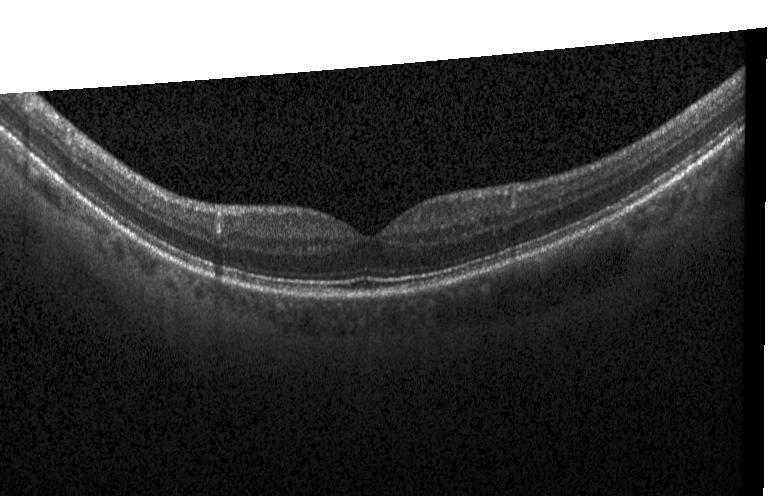
Retinal OCT B-scan · centered on the fovea · spectral-domain OCT. Macular OCT: no CNV, DME, or drusen.